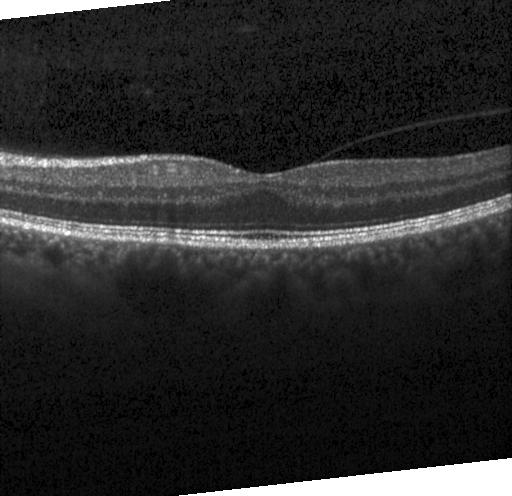
Centered on the fovea, retinal OCT B-scan.
Assessment: no CNV, DME, or drusen.